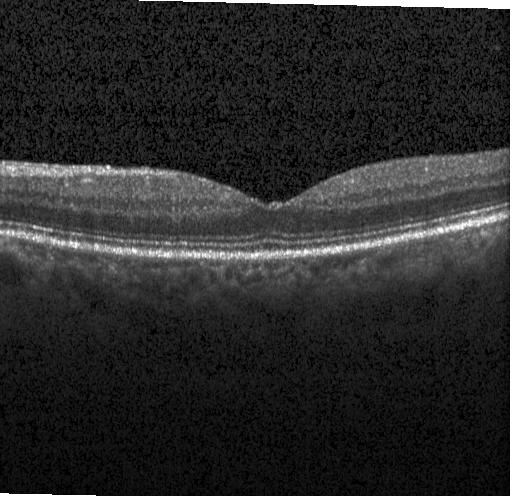
The scan shows no CNV, DME, or drusen.